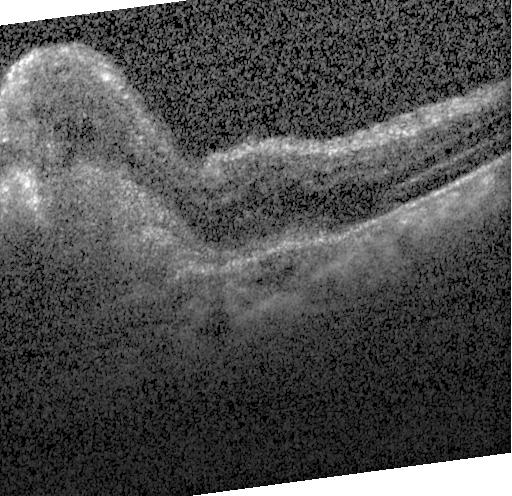 Diagnosis: a choroidal neovascular membrane.